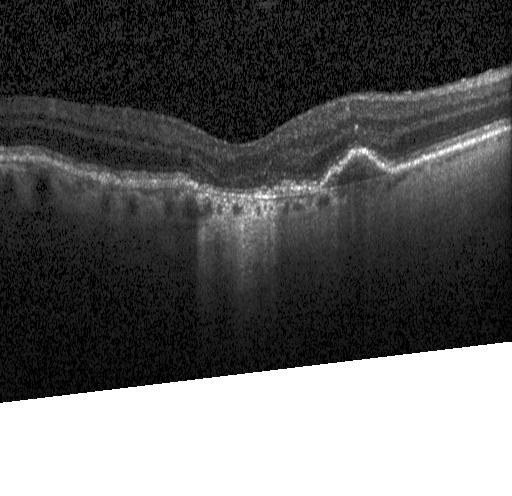
Optical coherence tomography scan — The scan shows CNV.